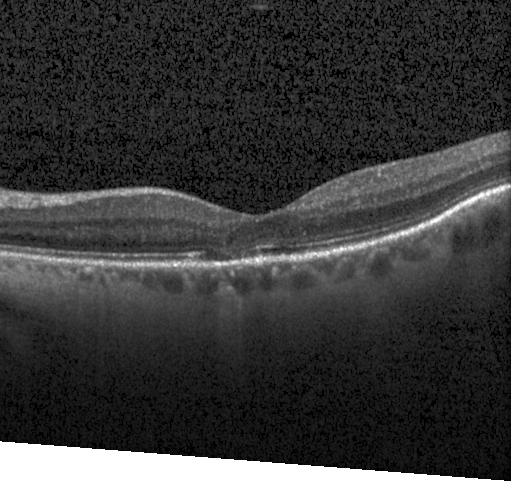
Optical coherence tomography scan · horizontal scan through the fovea · instrument: Heidelberg Spectralis — Assessment: no CNV, no DME, and no drusen.